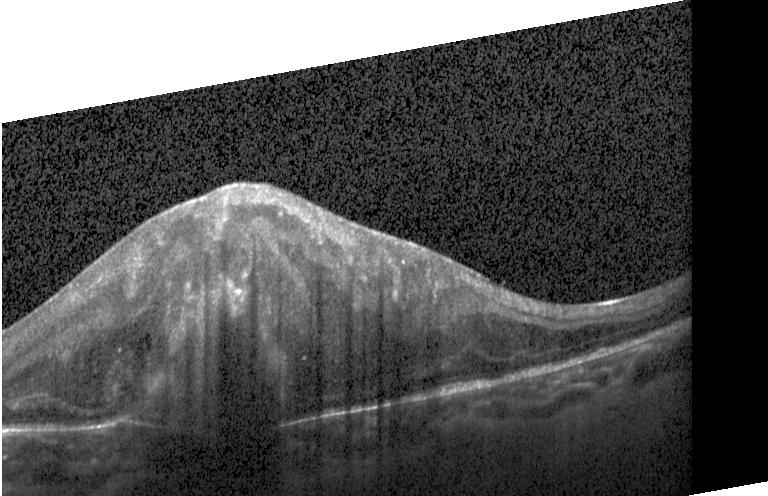

Macular OCT: a choroidal neovascular membrane.